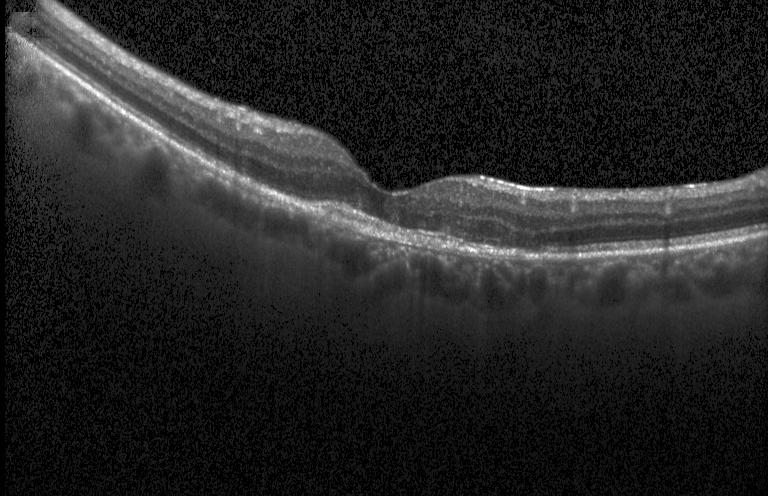 SD-OCT · through the macula · Heidelberg Spectralis · retinal OCT B-scan — Impression: a choroidal neovascular membrane.